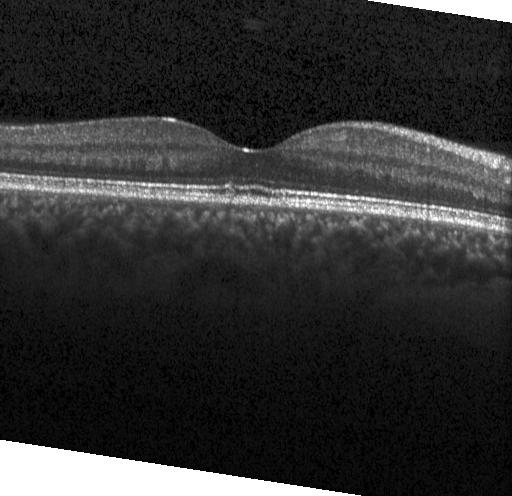
Spectral-domain optical coherence tomography; retinal OCT cross-section; horizontal scan through the fovea. Finding: no evidence of choroidal neovascularization, diabetic macular edema, or drusen.